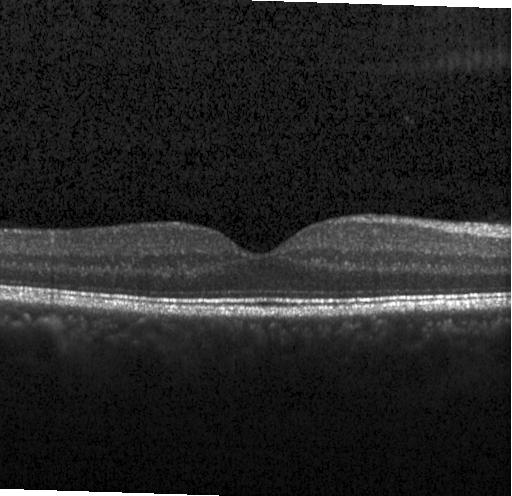

OCT scan showing no CNV, DME, or drusen.